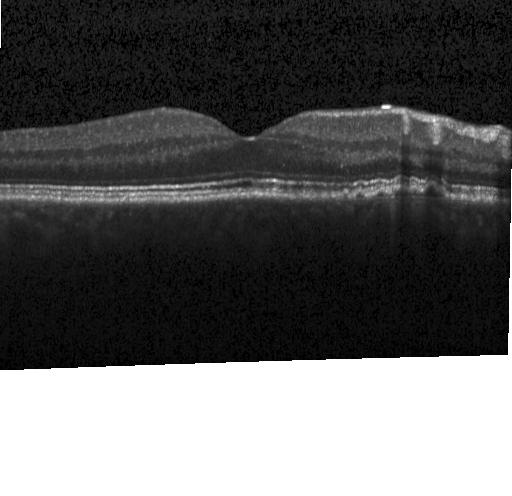

Macular OCT demonstrating choroidal neovascularization (CNV).